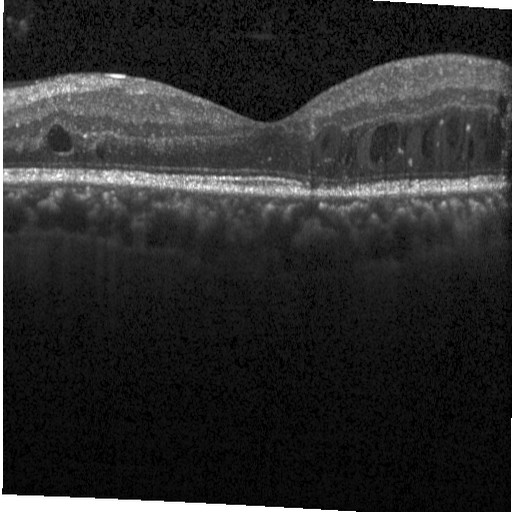 Impression: diabetic macular edema.